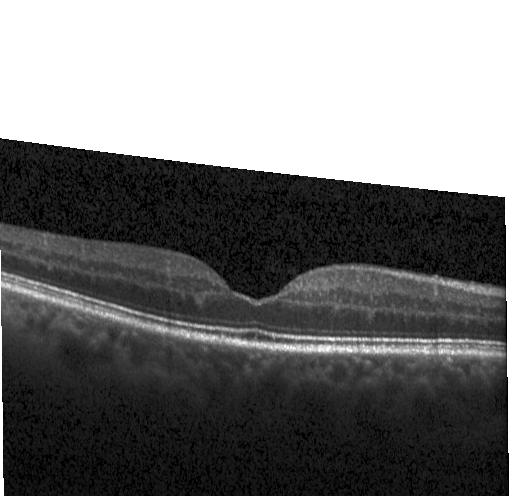

OCT line scan. Through the macula
Assessment: no choroidal neovascularization, diabetic macular edema, or drusen.